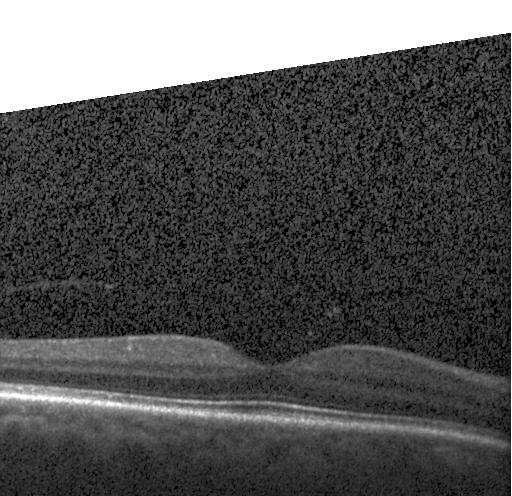

Through the macula · spectral-domain OCT · OCT B-scan · Heidelberg Spectralis.
Impression: no CNV, no DME, and no drusen.